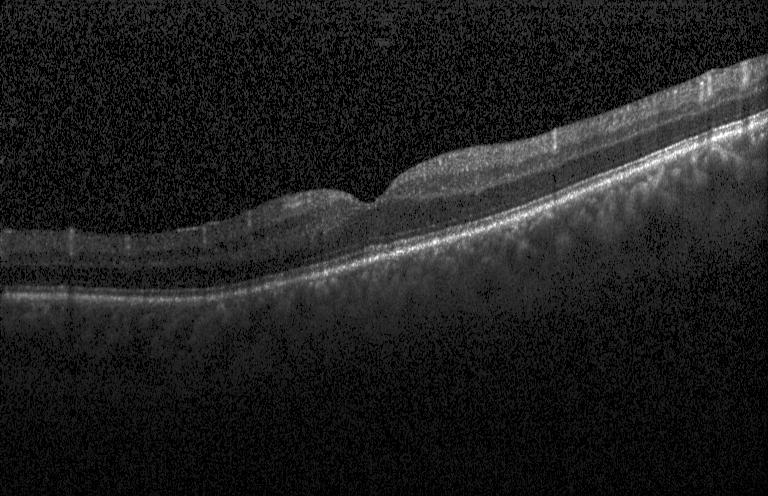
Diagnosis: no choroidal neovascularization, no diabetic macular edema, and no drusen.